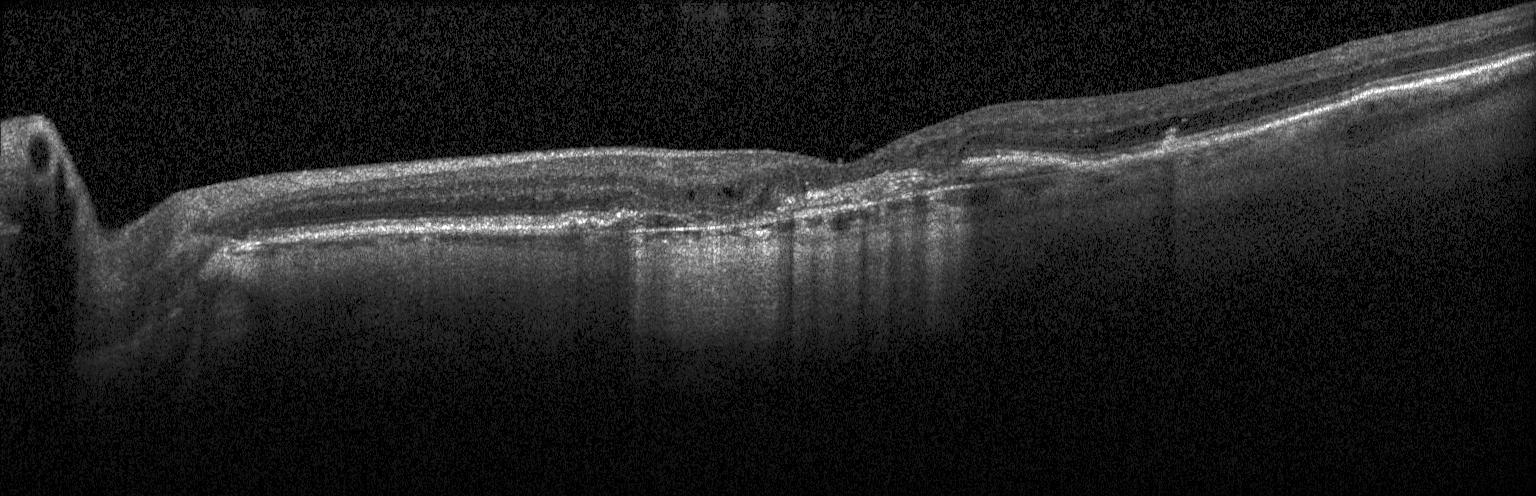
SD-OCT. Optical coherence tomography scan — Impression: choroidal neovascularization (CNV).